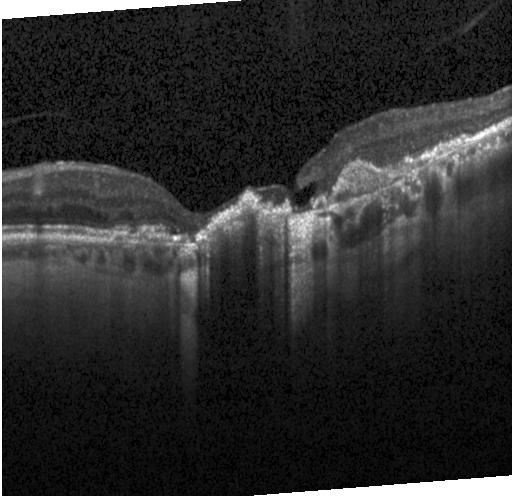 Acquired on a Heidelberg Spectralis; centered on the fovea; SD-OCT; OCT line scan. Finding: choroidal neovascularization (CNV).